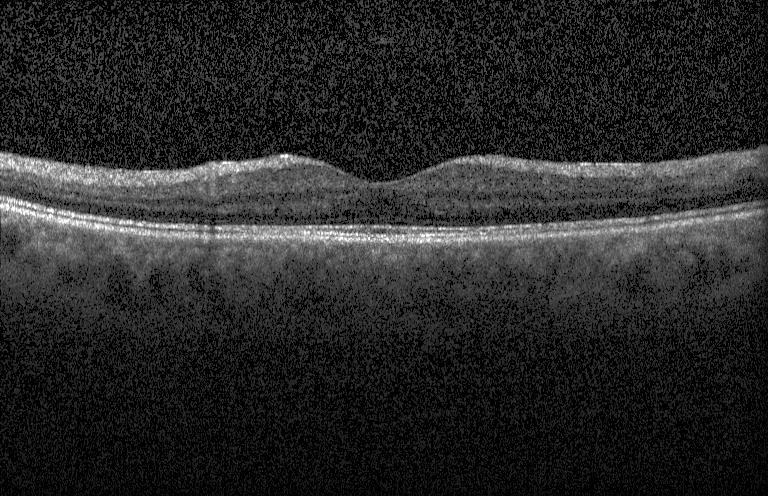

Diagnosis: no choroidal neovascularization, no diabetic macular edema, and no drusen.